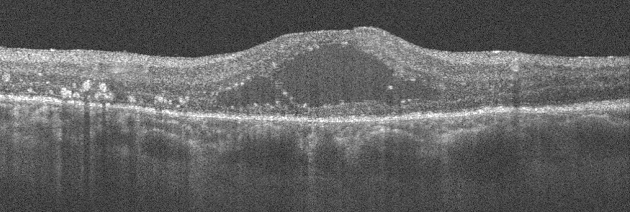

Macular OCT: DME.